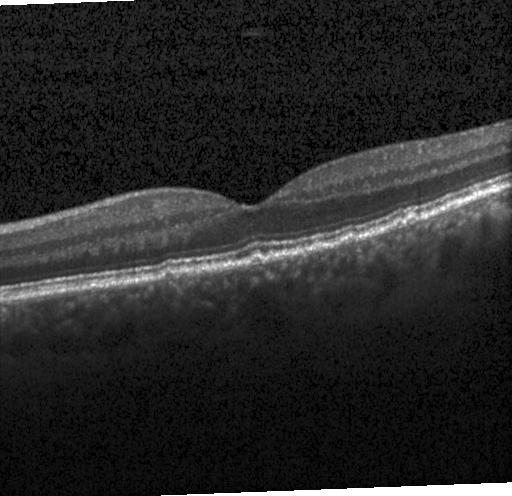 Diagnosis: sub-RPE drusenoid deposits.